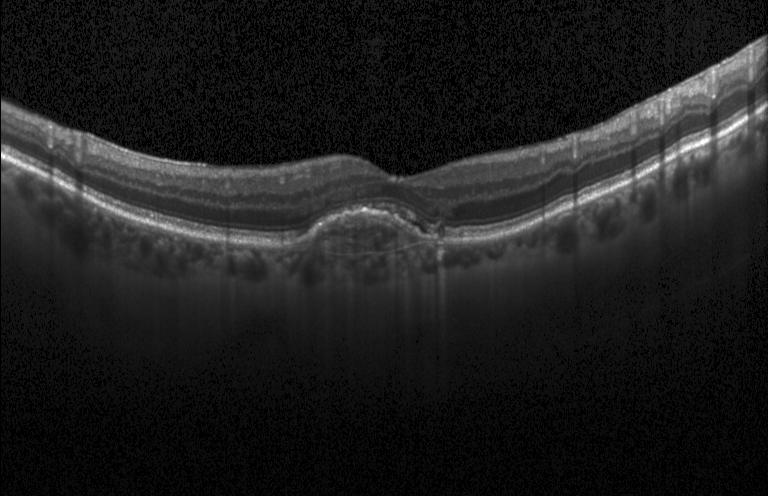 Finding: choroidal neovascularization (CNV).